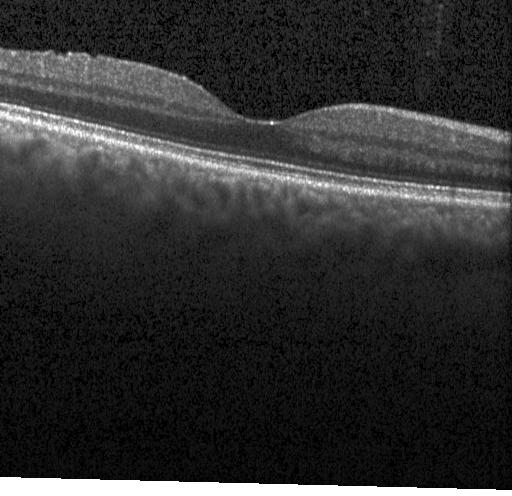 Fovea-centered; optical coherence tomography B-scan — Macular OCT: no CNV, DME, or drusen.